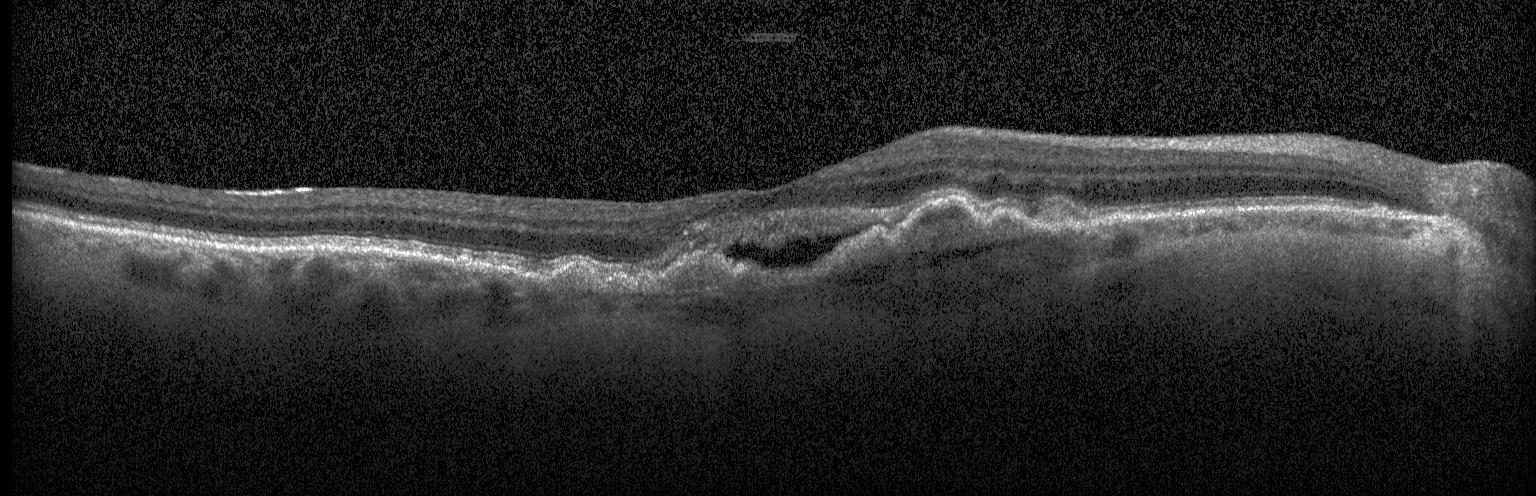
Optical coherence tomography scan — Macular OCT: a choroidal neovascular membrane.